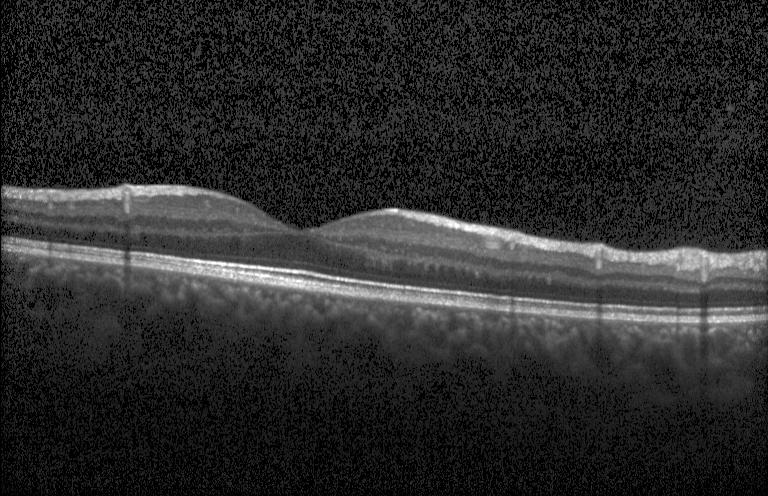

Spectral-domain OCT B-scan: no CNV, DME, or drusen.